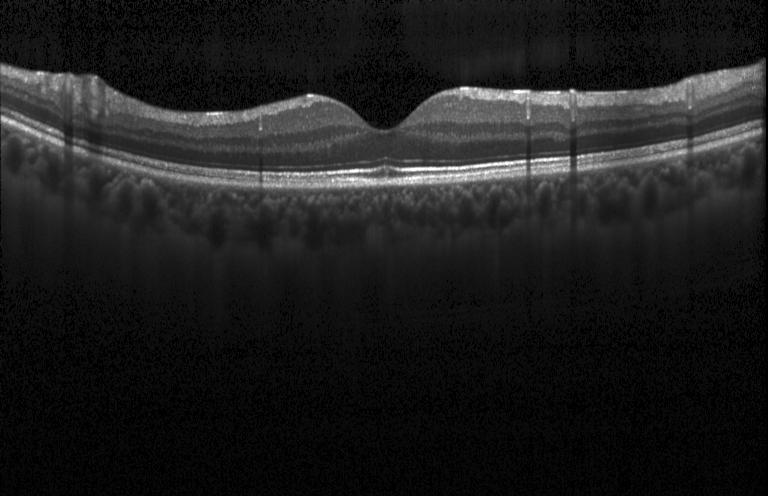

Retinal OCT B-scan — Diagnosis: no choroidal neovascularization, no diabetic macular edema, and no drusen.